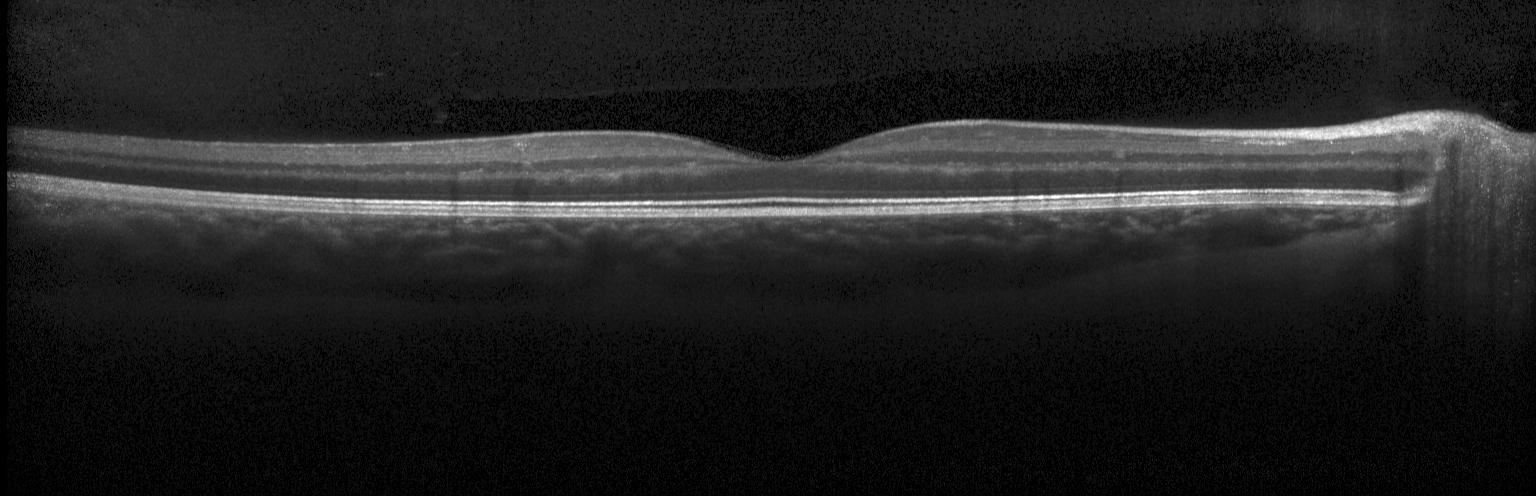
The scan shows no evidence of choroidal neovascularization, diabetic macular edema, or drusen.